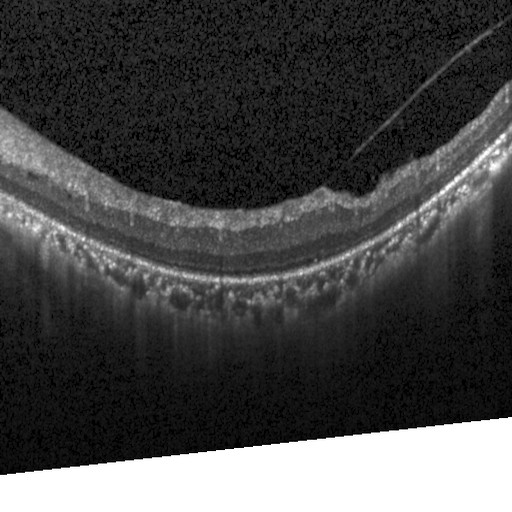 OCT B-scan · SD-OCT · fovea-centered — The scan shows diabetic macular edema (DME).